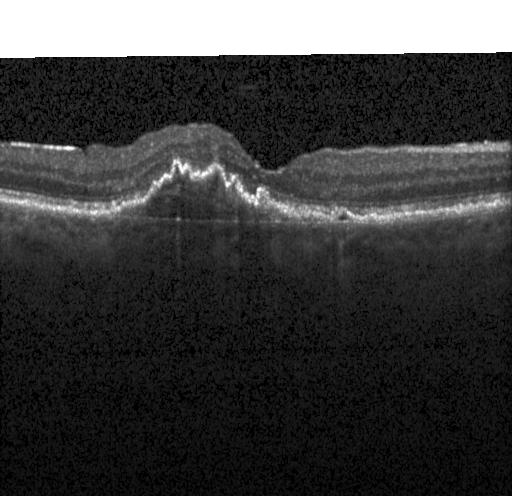
Optical coherence tomography scan.
Impression: a choroidal neovascular membrane.